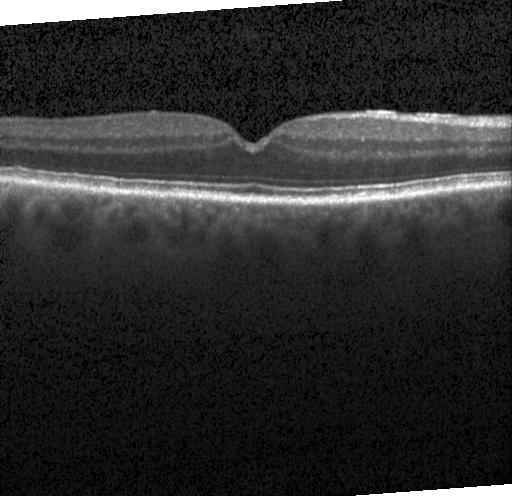
Retinal OCT cross-section.
This B-scan demonstrates no CNV, no DME, and no drusen.